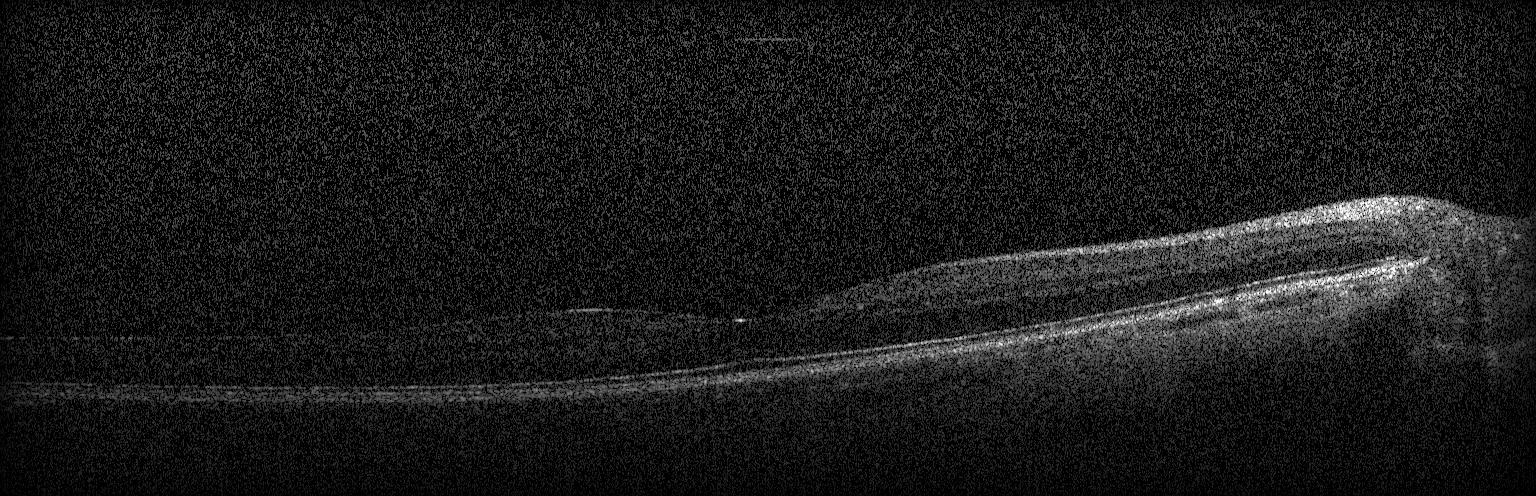

OCT B-scan — Diagnosis: no evidence of choroidal neovascularization, diabetic macular edema, or drusen.